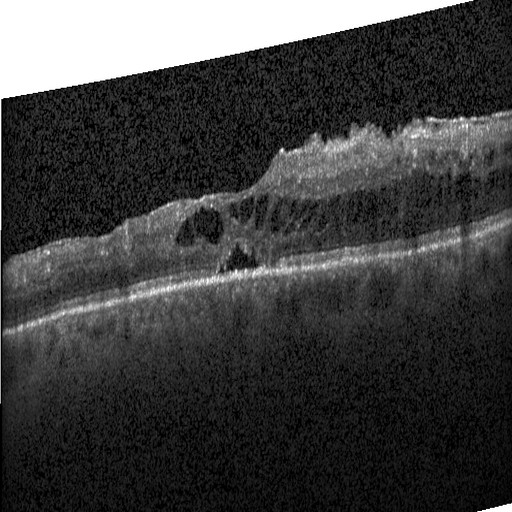 Impression: DME.